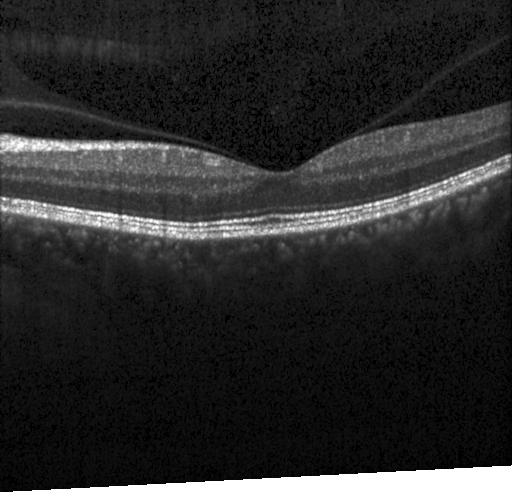

Neither CNV, DME, nor drusen.